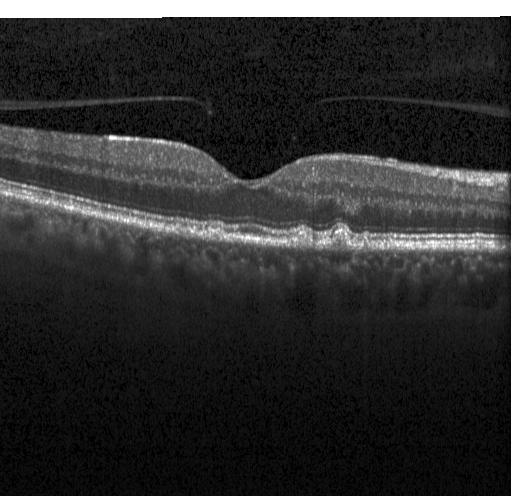 Dx: drusen.